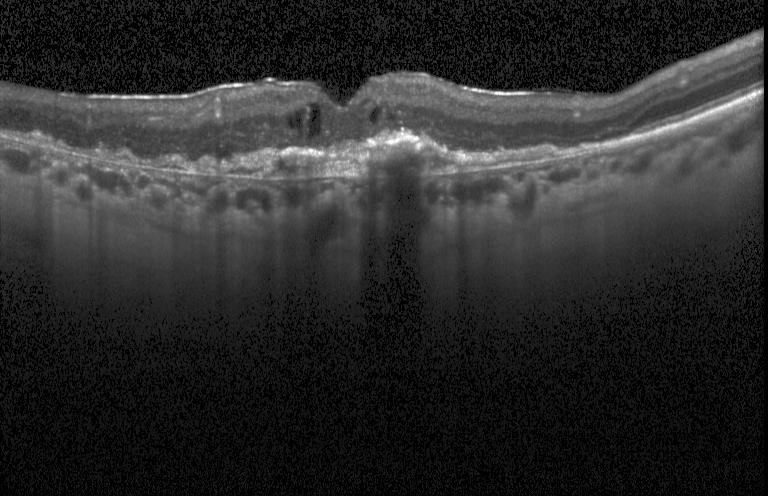

Finding: a choroidal neovascular membrane.